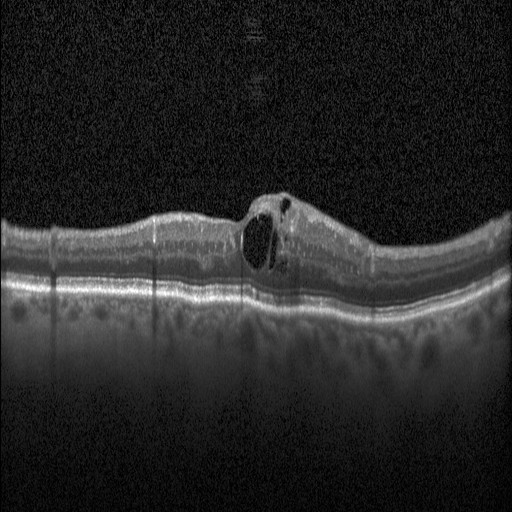
Centered on the fovea, retinal OCT B-scan. OCT finding: diabetic macular edema.